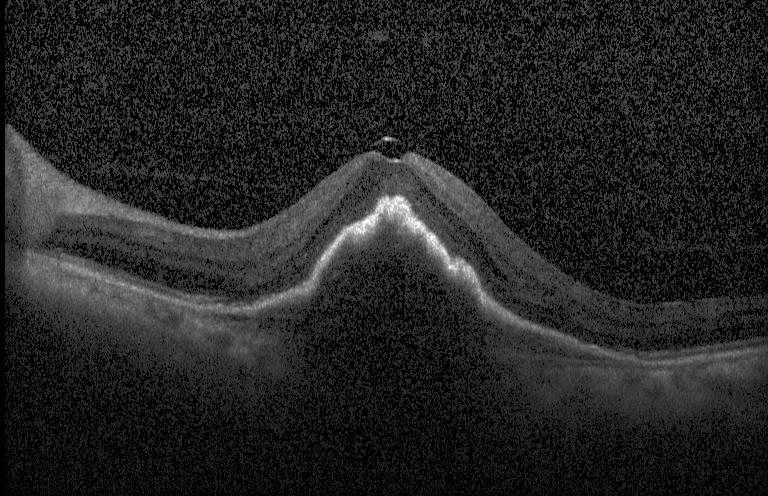

Diagnosis: choroidal neovascularization (CNV).